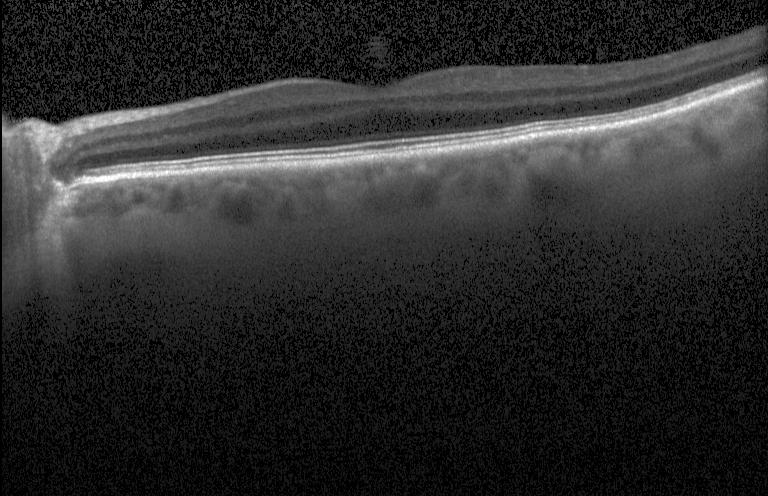
Retinal OCT cross-section showing no choroidal neovascularization, diabetic macular edema, or drusen.